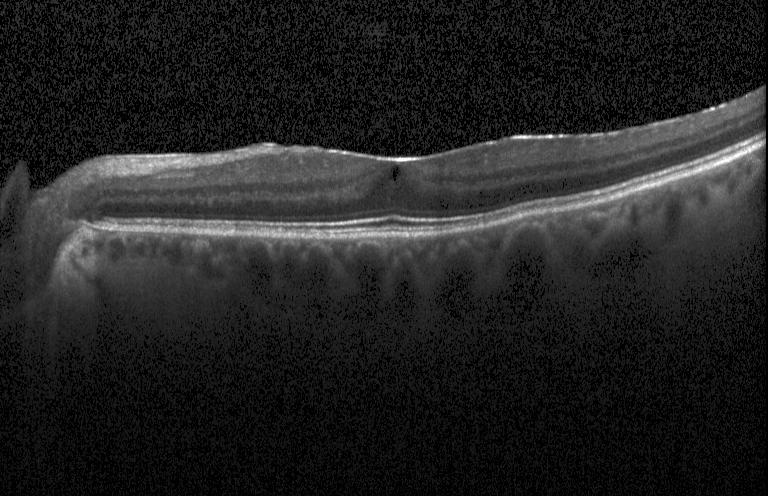 DME.